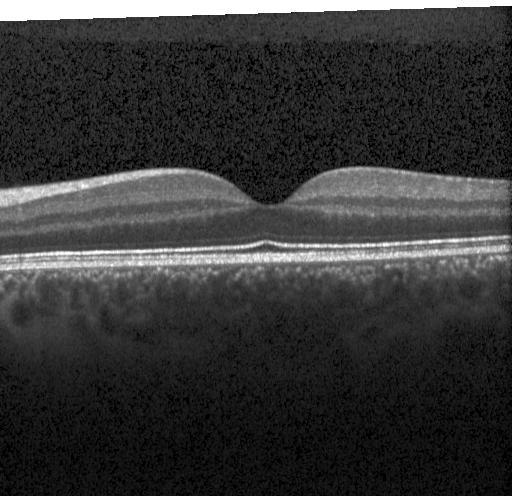 Finding: no evidence of choroidal neovascularization, diabetic macular edema, or drusen.